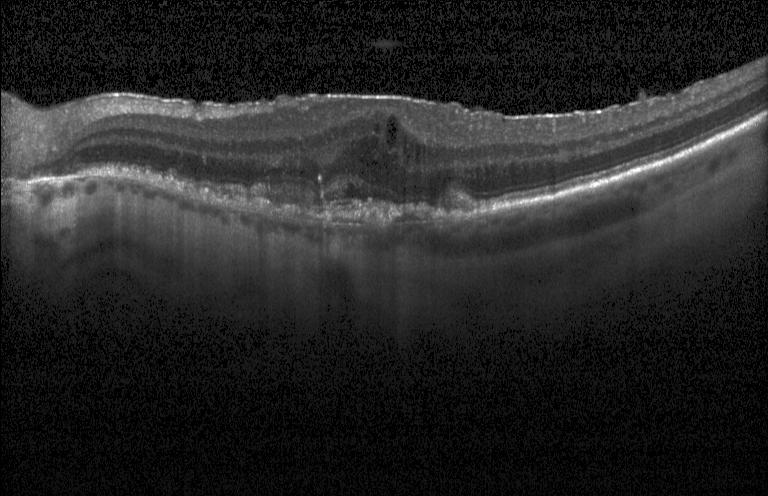

Retinal OCT cross-section — This B-scan demonstrates choroidal neovascularization.